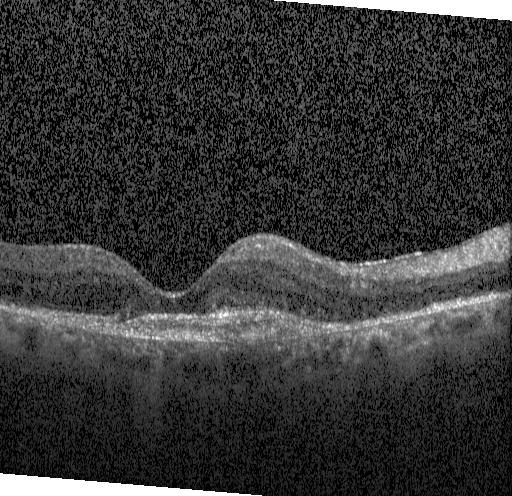

Instrument: Heidelberg Spectralis; OCT line scan. Impression: choroidal neovascularization.